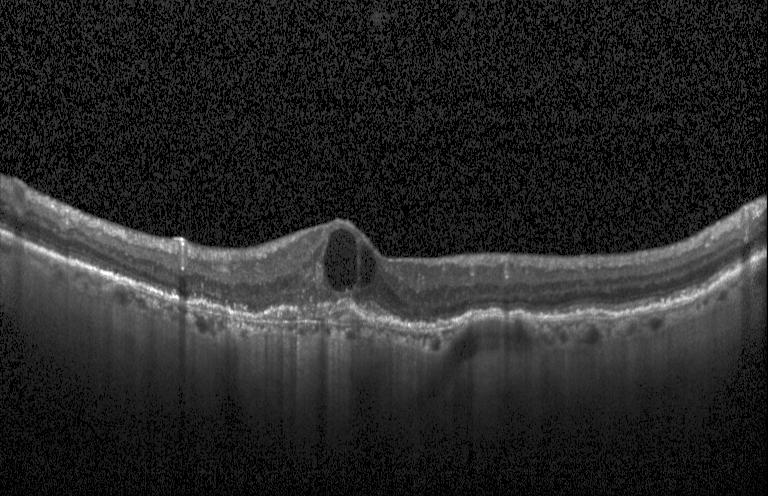

Optical coherence tomography B-scan; centered on the fovea
Macular OCT: a choroidal neovascular membrane.